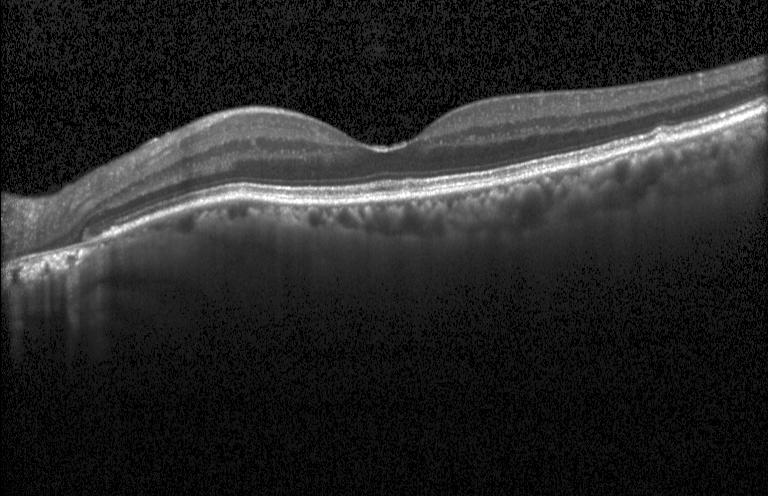 SD-OCT, retinal OCT cross-section. Finding: no choroidal neovascularization, diabetic macular edema, or drusen.